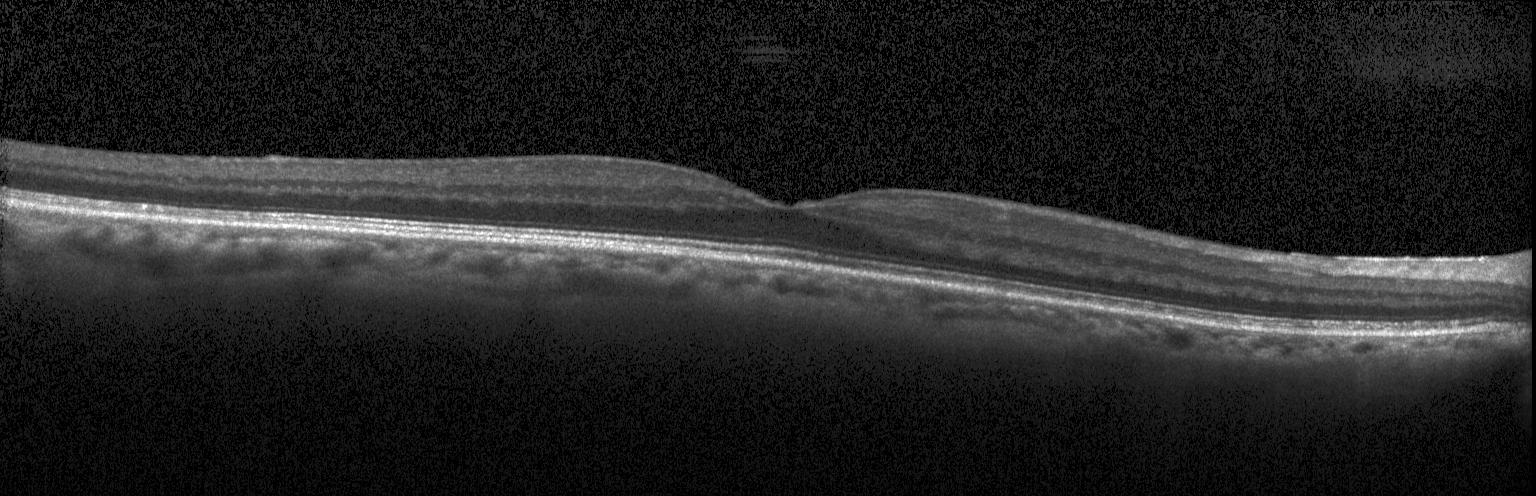

This B-scan demonstrates no choroidal neovascularization, diabetic macular edema, or drusen.